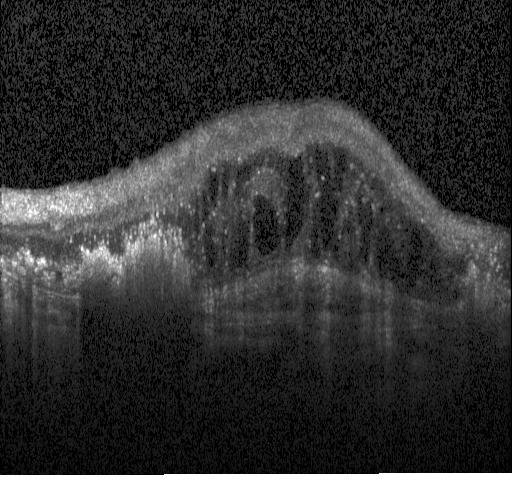

SD-OCT · through the macula · optical coherence tomography B-scan.
Macular OCT: diabetic macular edema (DME).